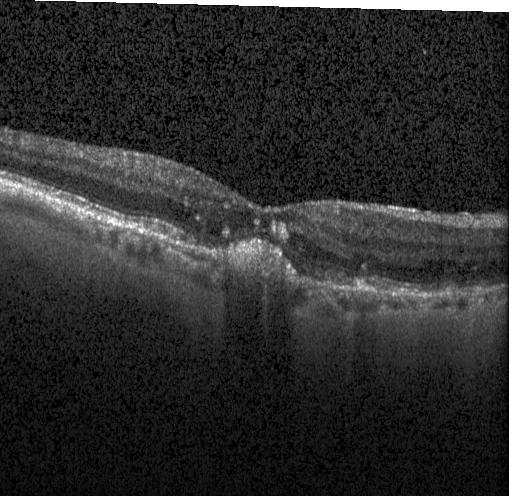 OCT B-scan showing a choroidal neovascular membrane.